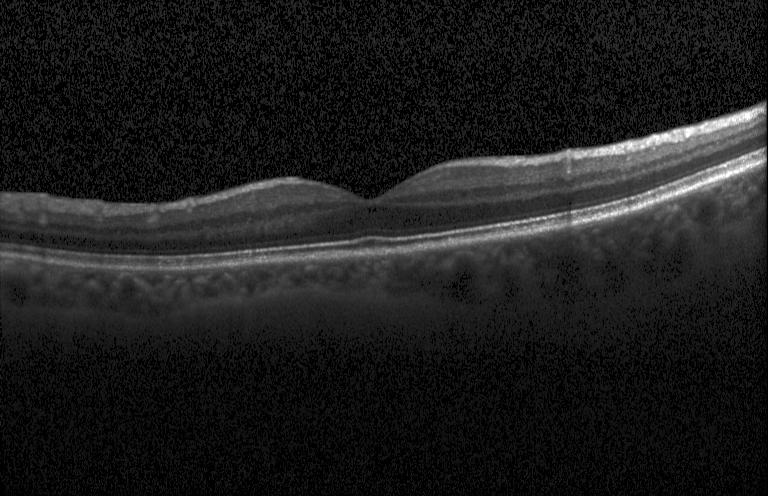 No CNV, DME, or drusen.